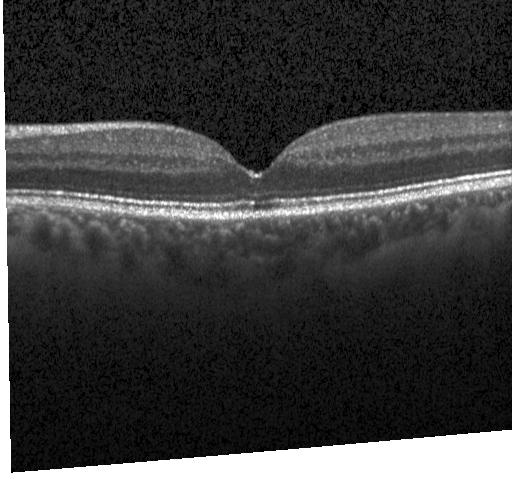

Retinal OCT B-scan; spectral-domain OCT; Heidelberg Spectralis OCT system. Macular OCT: no evidence of choroidal neovascularization, diabetic macular edema, or drusen.